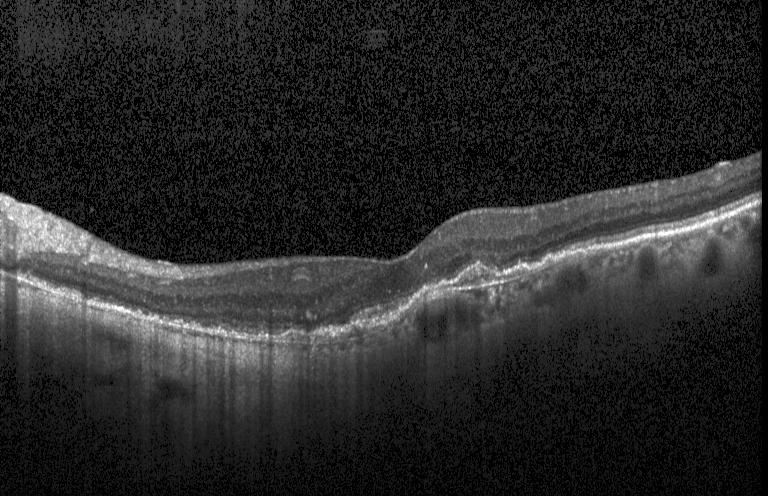

OCT B-scan showing a choroidal neovascular membrane.